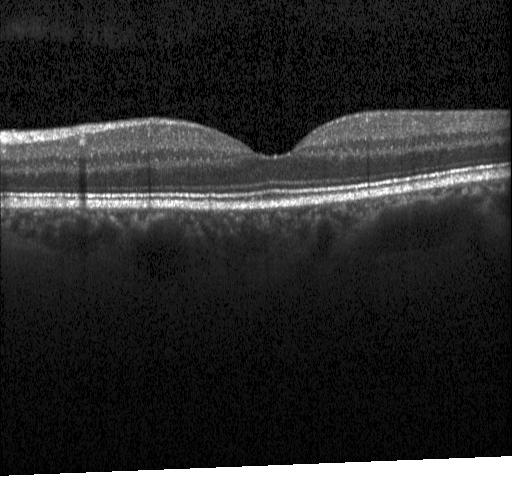
OCT line scan
Impression: no evidence of choroidal neovascularization, diabetic macular edema, or drusen.